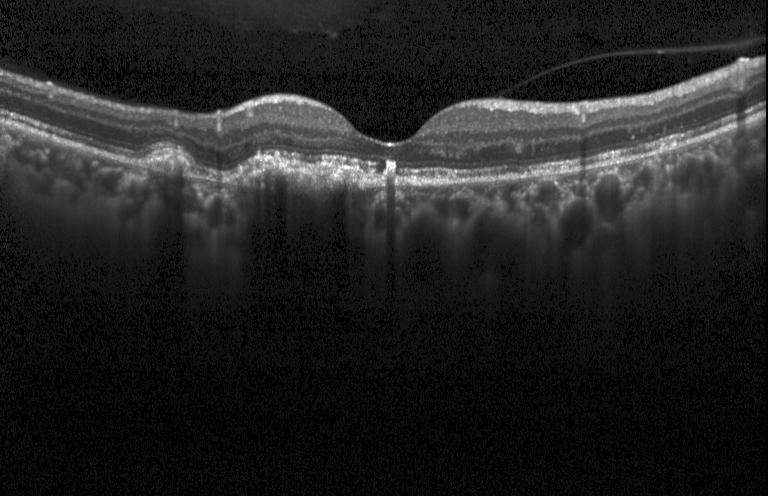 Choroidal neovascularization (CNV).